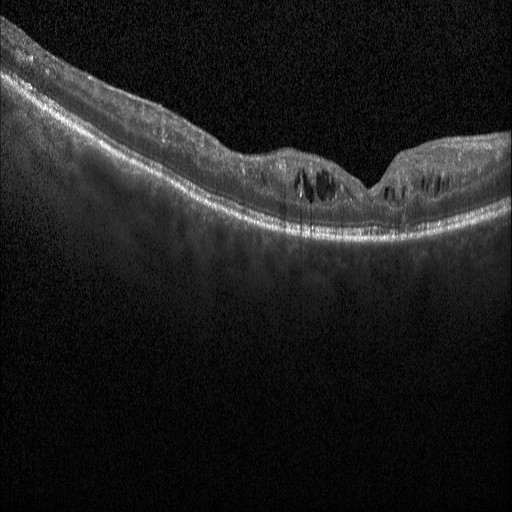
Impression: diabetic macular edema (DME).